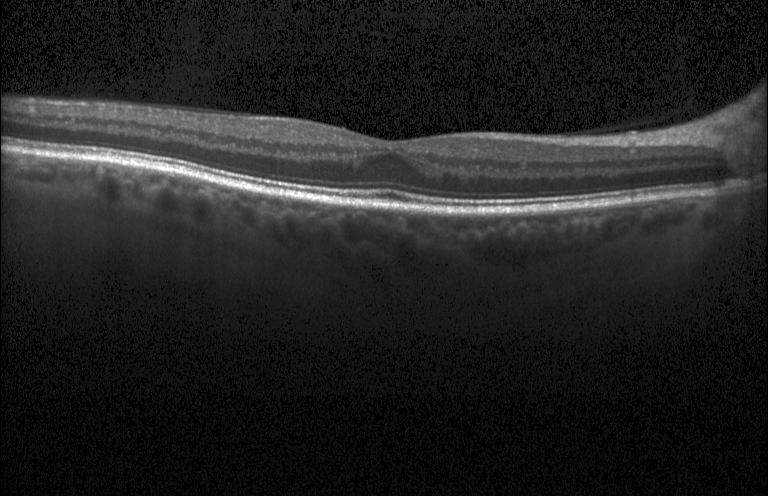
OCT finding: no CNV, no DME, and no drusen.